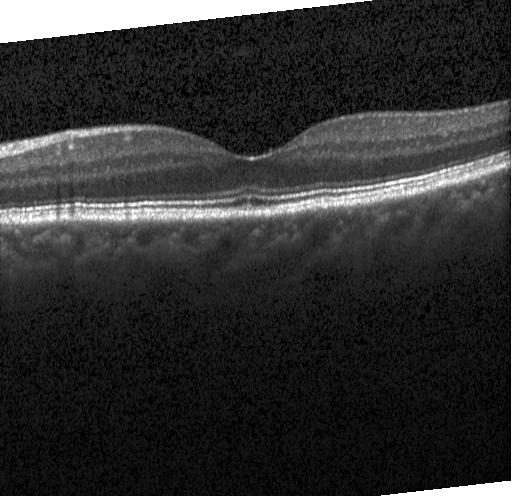 Centered on the fovea, instrument: Heidelberg Spectralis, retinal OCT B-scan, spectral-domain optical coherence tomography.
Neither choroidal neovascularization, diabetic macular edema, nor drusen.